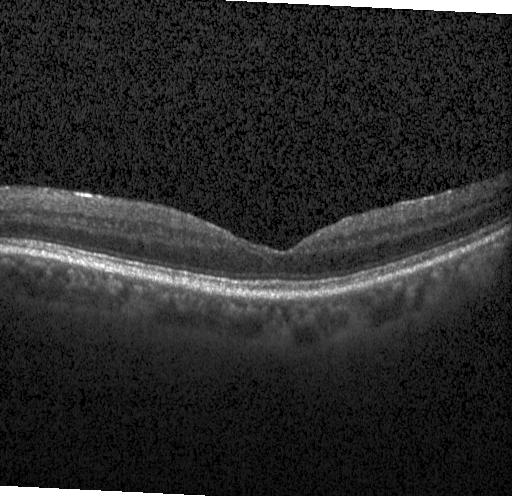 Finding: no choroidal neovascularization, no diabetic macular edema, and no drusen.